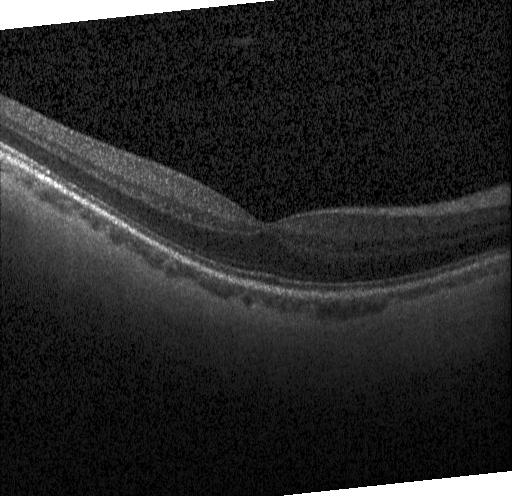
SD-OCT. Horizontal scan through the fovea. OCT B-scan. Heidelberg Spectralis OCT system.
This B-scan demonstrates no choroidal neovascularization, diabetic macular edema, or drusen.